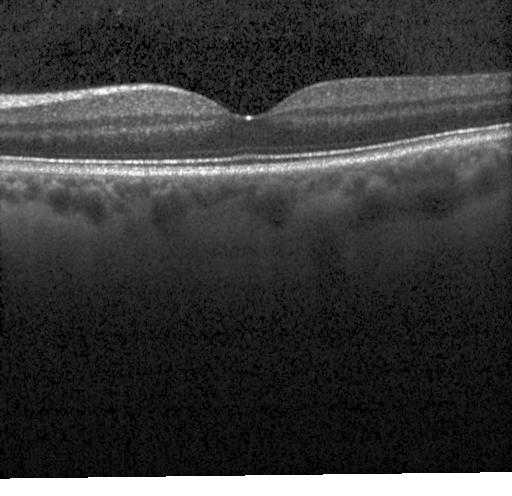
Optical coherence tomography B-scan. Macular OCT: no evidence of CNV, DME, or drusen.